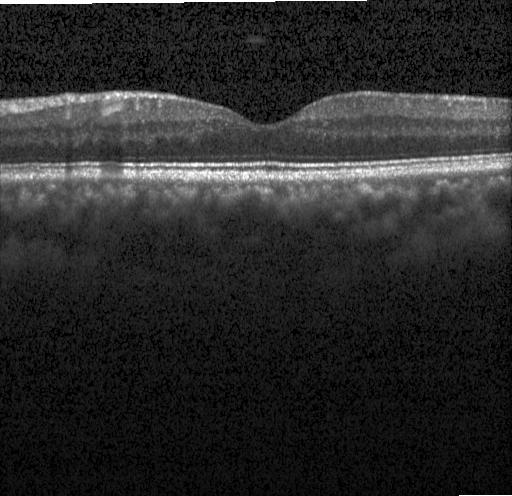 Centered on the fovea · spectral-domain OCT · Heidelberg Spectralis · OCT B-scan. Diagnosis: no CNV, DME, or drusen.